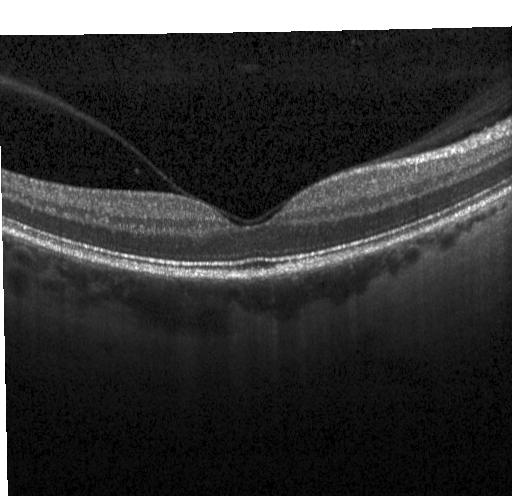
Horizontal scan through the fovea · spectral-domain OCT · Heidelberg Spectralis OCT system · retinal OCT cross-section — Dx: neither CNV, DME, nor drusen.